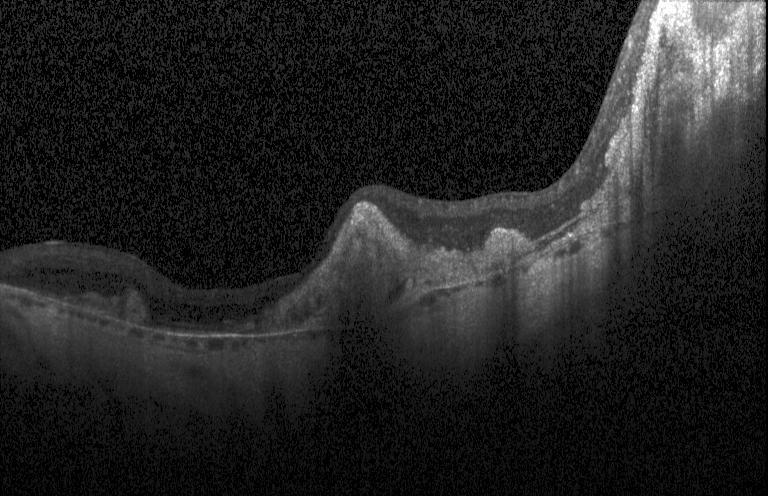

OCT line scan, SD-OCT, fovea-centered. Finding: a choroidal neovascular membrane.